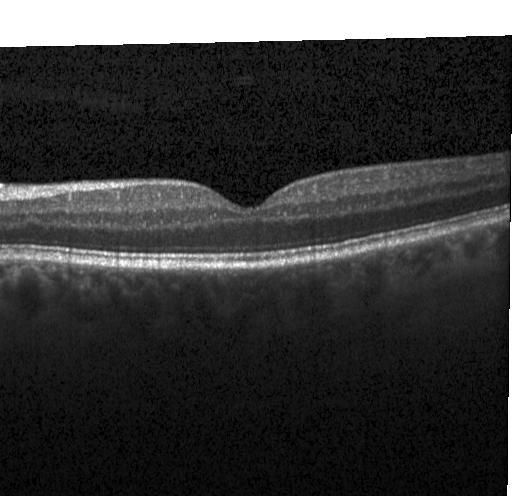 Assessment: neither CNV, DME, nor drusen.